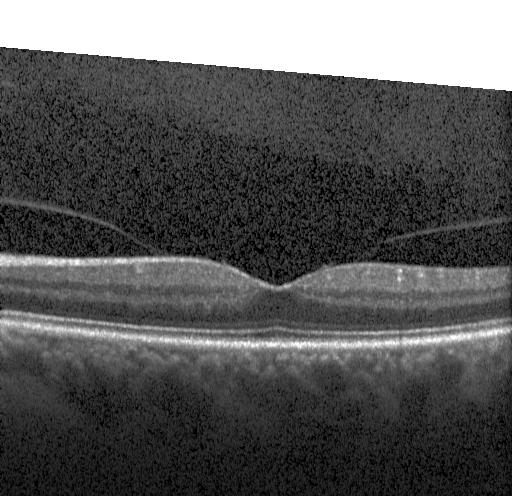

This B-scan demonstrates no choroidal neovascularization, no diabetic macular edema, and no drusen.